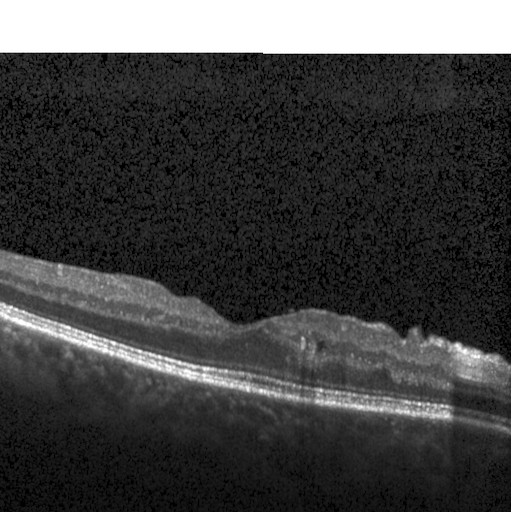

Retinal OCT cross-section, centered on the fovea, Heidelberg Spectralis — Impression: diabetic macular edema.